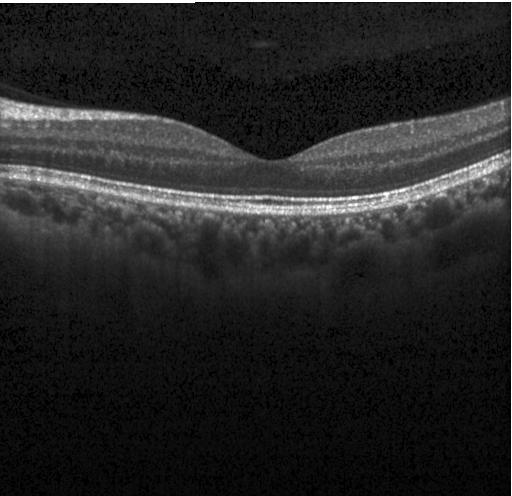

Fovea-centered; SD-OCT; retinal OCT B-scan
The scan shows no evidence of choroidal neovascularization, diabetic macular edema, or drusen.